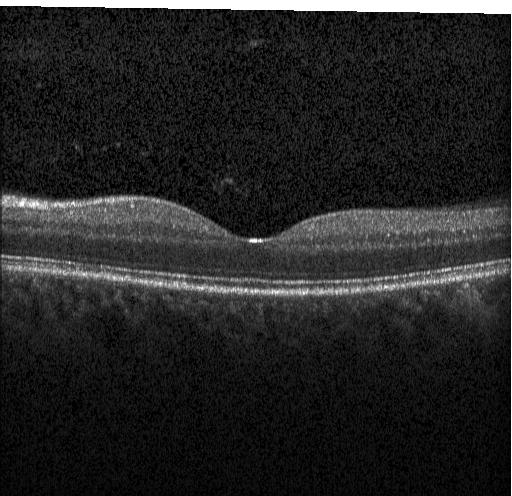 Diagnosis: no choroidal neovascularization, no diabetic macular edema, and no drusen.